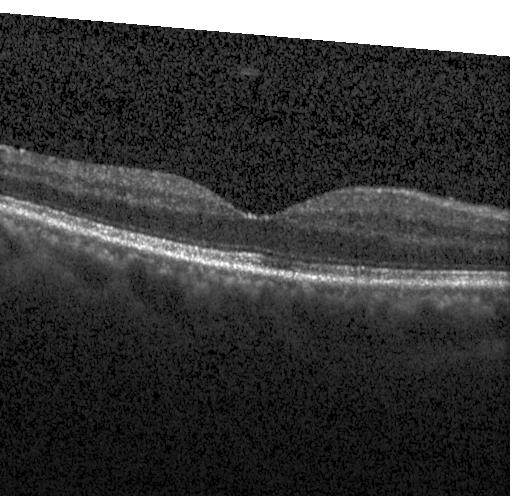

Macular OCT: no evidence of choroidal neovascularization, diabetic macular edema, or drusen.